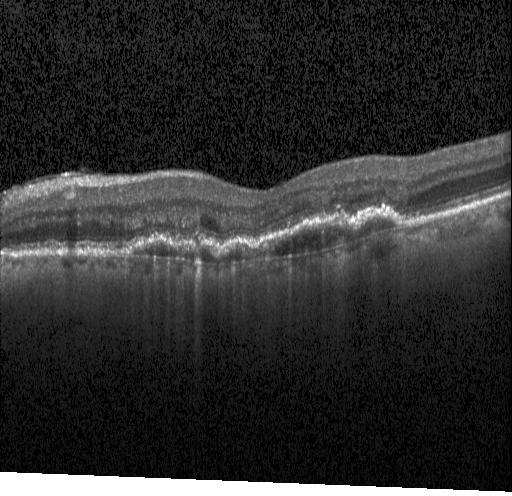
OCT line scan · fovea-centered · Heidelberg Spectralis.
Macular OCT: choroidal neovascularization.